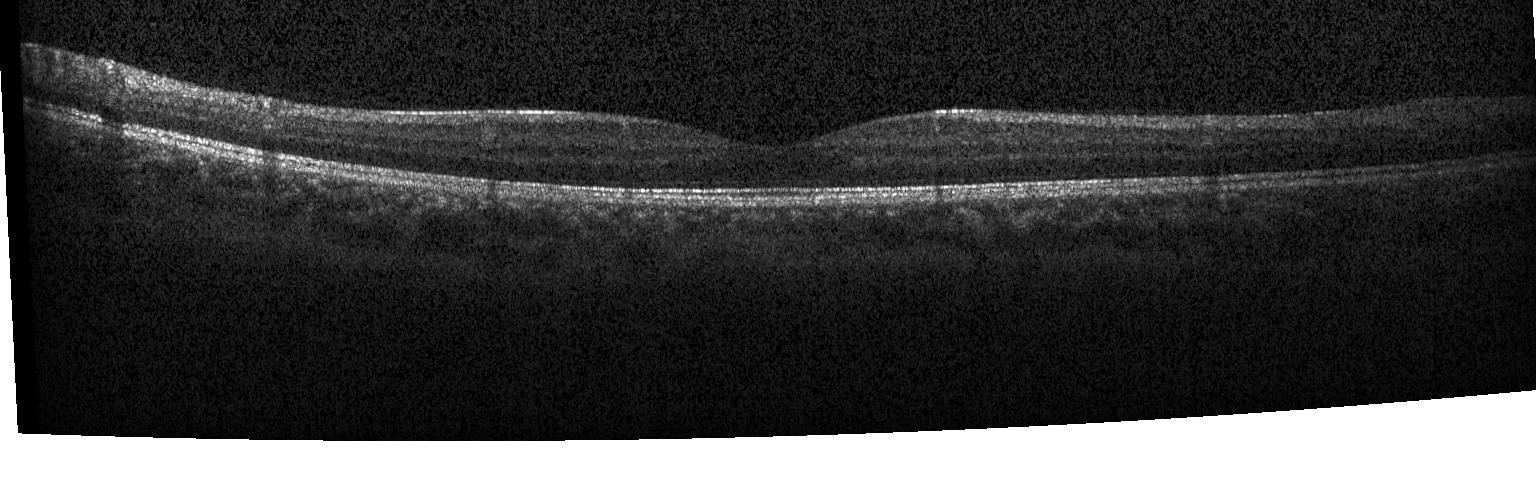

Optical coherence tomography B-scan — Diagnosis: no choroidal neovascularization, no diabetic macular edema, and no drusen.